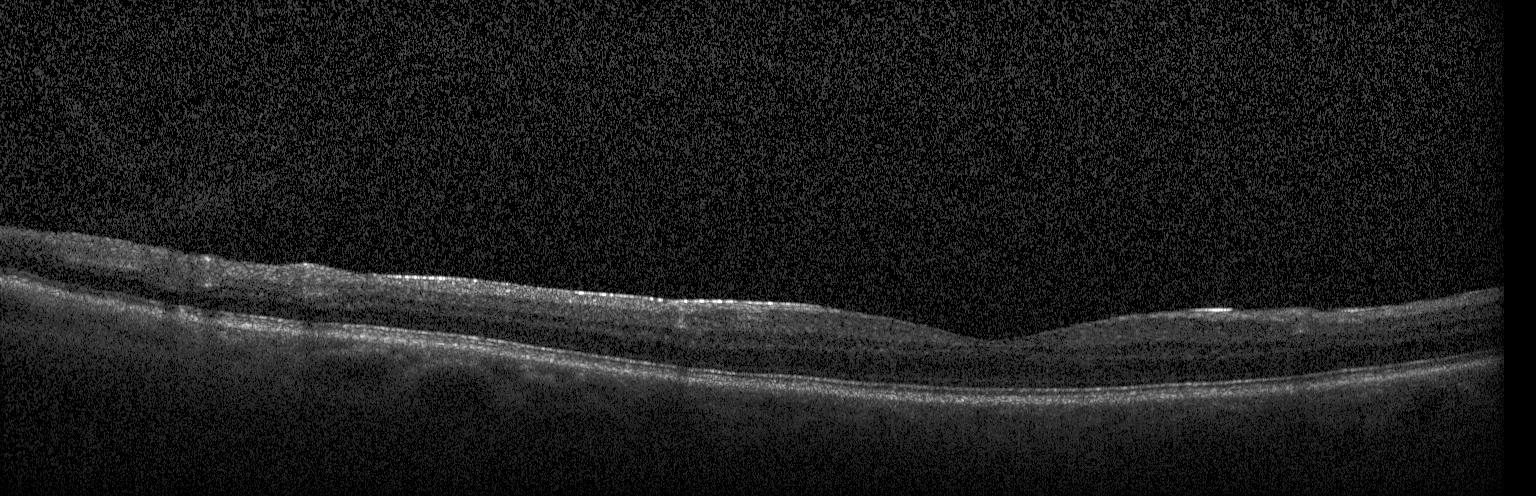 Heidelberg Spectralis OCT system. Spectral-domain OCT. Retinal OCT cross-section. Fovea-centered. Macular OCT: neither choroidal neovascularization, diabetic macular edema, nor drusen.